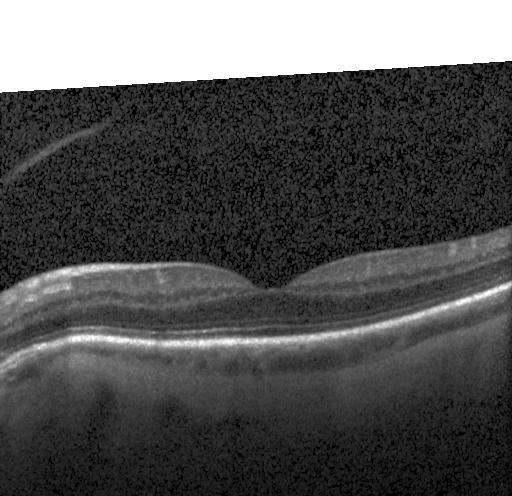

Retinal OCT B-scan. Macular scan.
Diagnosis: no choroidal neovascularization, diabetic macular edema, or drusen.